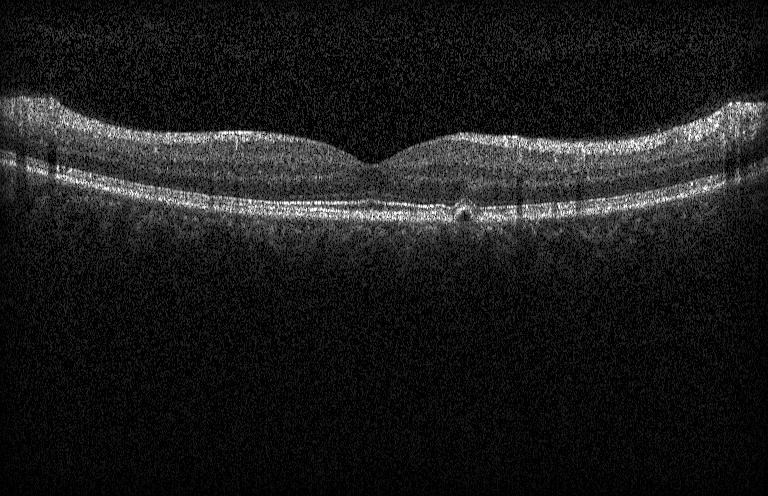 Retinal OCT cross-section.
Macular OCT: drusen.